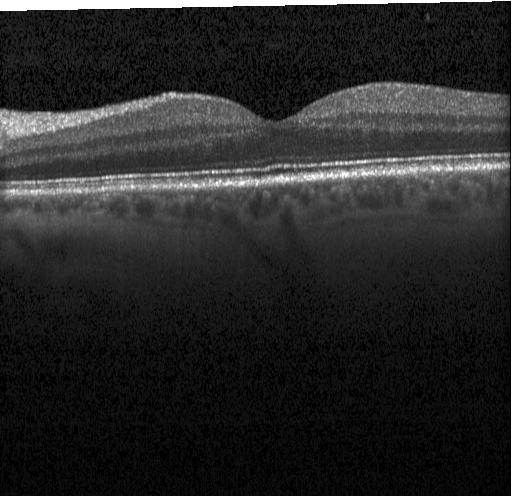

Macular OCT: no choroidal neovascularization, no diabetic macular edema, and no drusen.